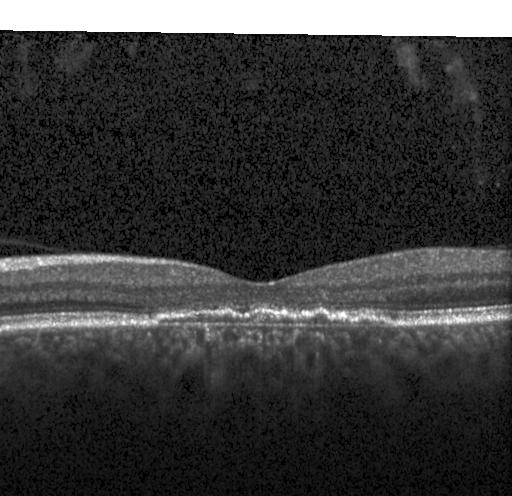

Finding: a choroidal neovascular membrane.